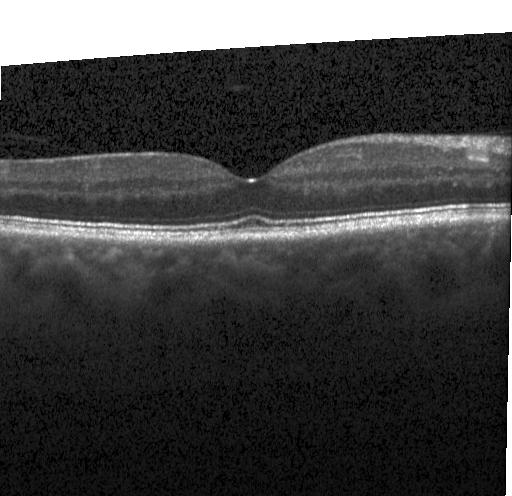

Impression: no CNV, DME, or drusen.